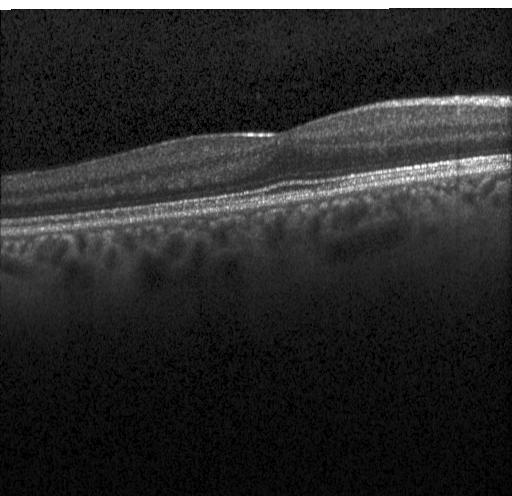 Dx: no evidence of CNV, DME, or drusen.